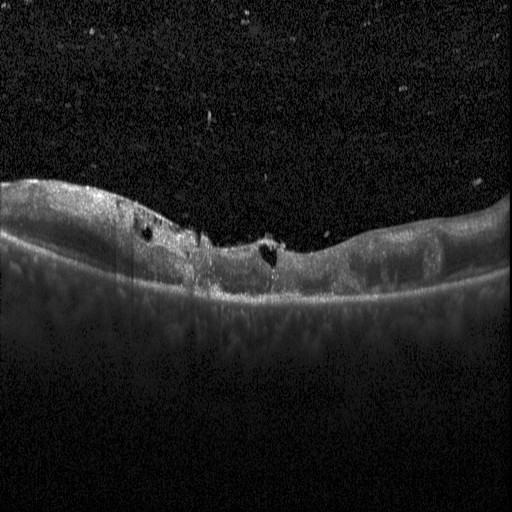

OCT B-scan showing diabetic macular edema.